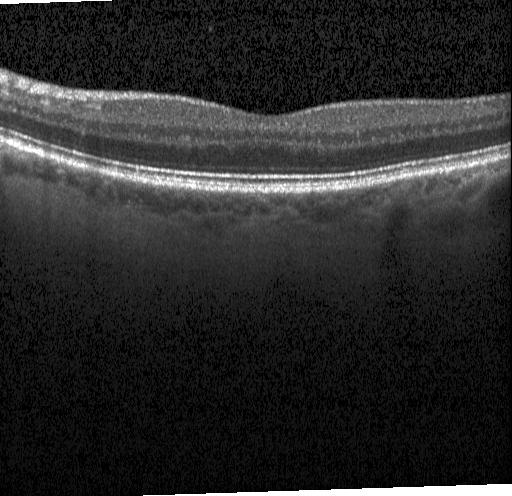
Spectral-domain OCT B-scan: no choroidal neovascularization, no diabetic macular edema, and no drusen.